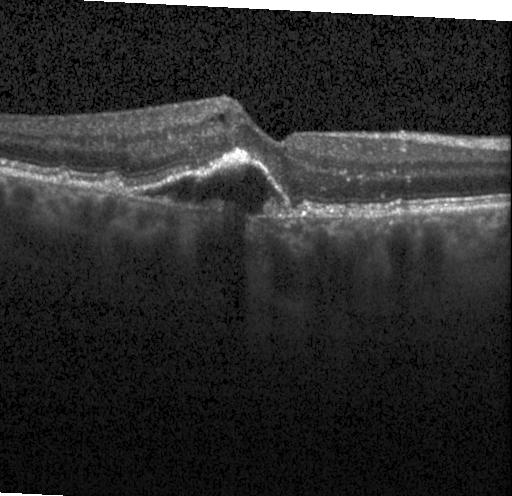 Dx: choroidal neovascularization.